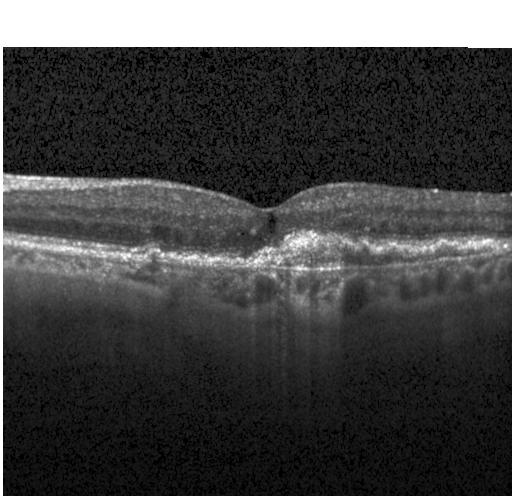
Centered on the fovea; spectral-domain OCT; retinal OCT B-scan — Assessment: a choroidal neovascular membrane.